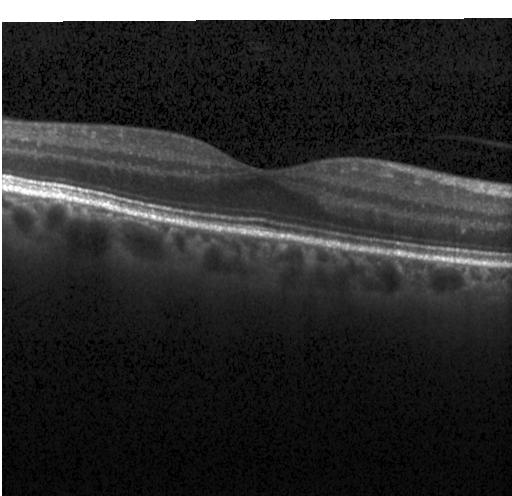

Through the macula; retinal OCT cross-section — Finding: neither CNV, DME, nor drusen.